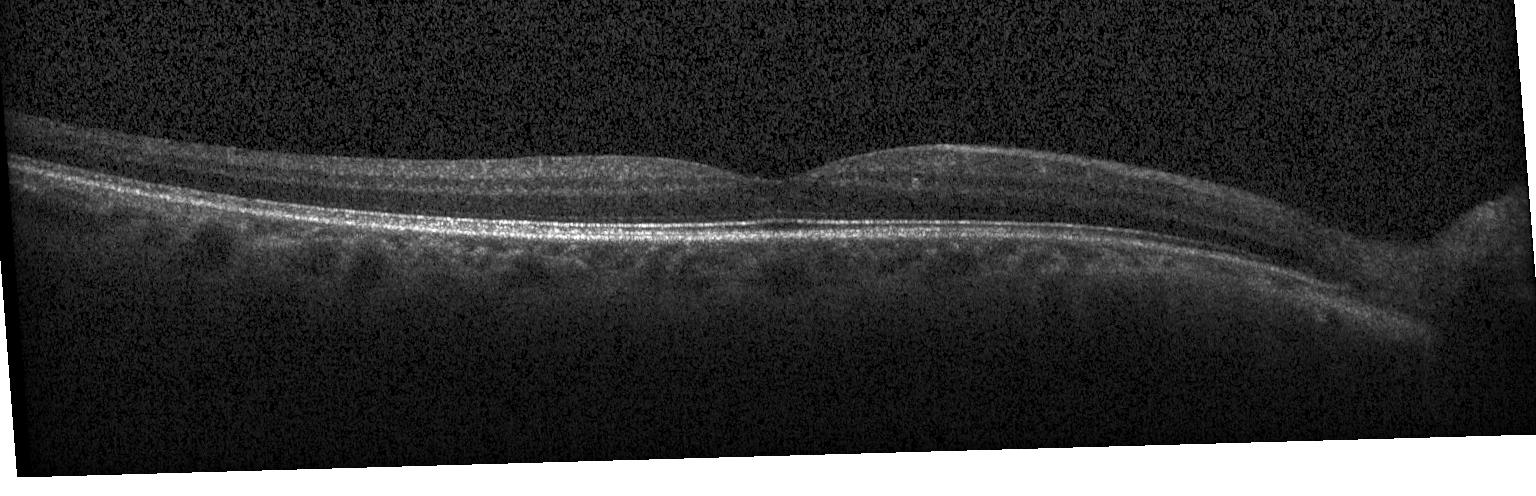
Centered on the fovea; Heidelberg Spectralis; SD-OCT; retinal OCT cross-section — Macular OCT: no CNV, DME, or drusen.